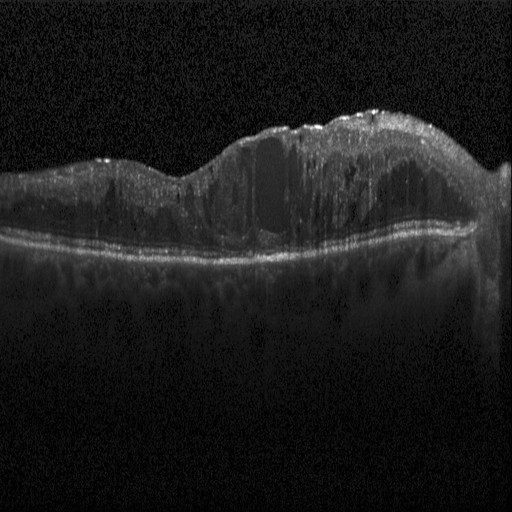
Assessment: DME.